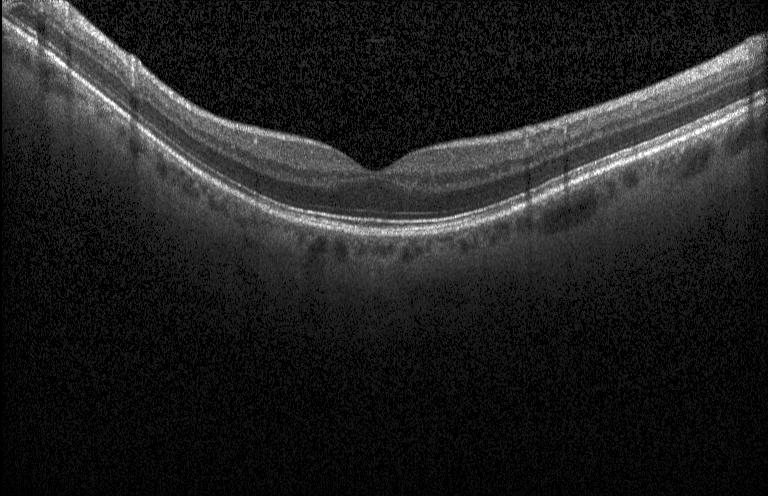 Through the macula. Optical coherence tomography scan
No choroidal neovascularization, diabetic macular edema, or drusen.